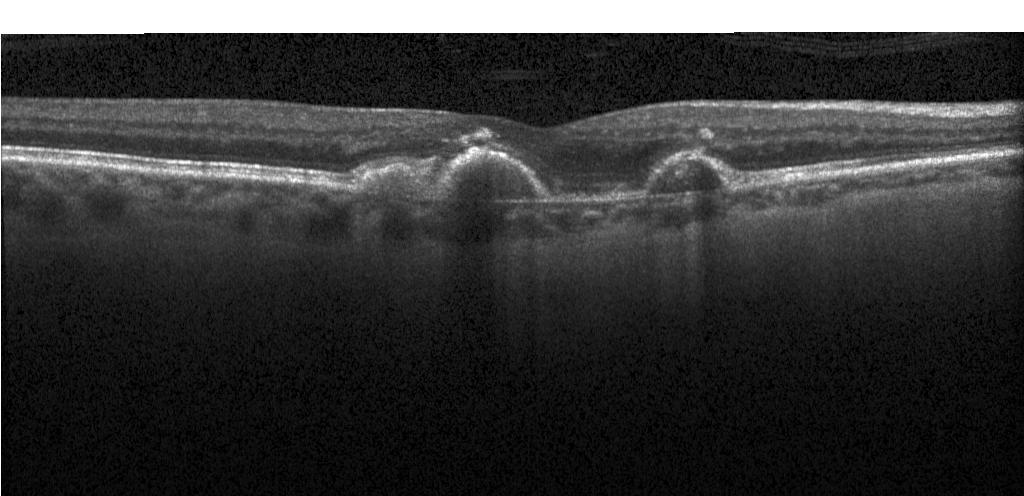
OCT B-scan showing a choroidal neovascular membrane.